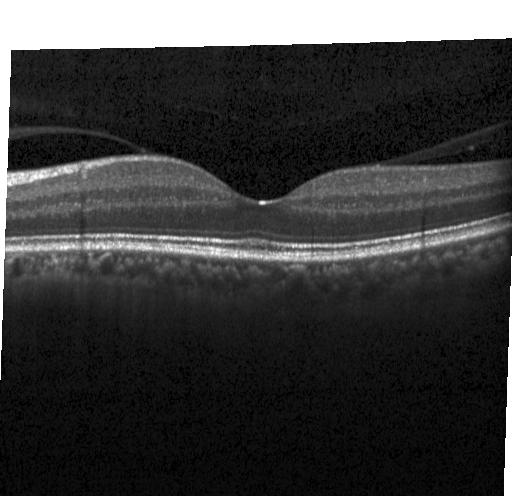 Heidelberg Spectralis, centered on the fovea, retinal OCT cross-section, spectral-domain OCT
Finding: neither CNV, DME, nor drusen.